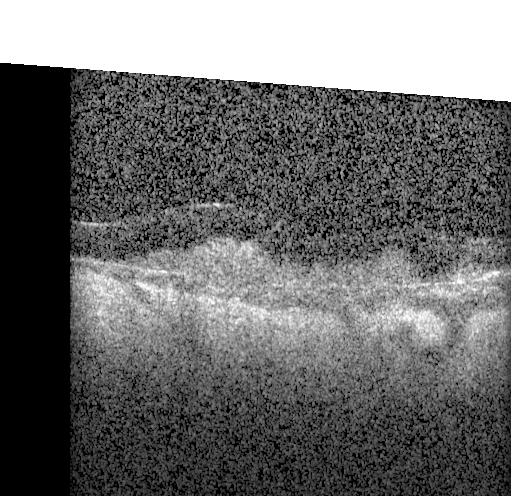 Acquired on a Heidelberg Spectralis. OCT line scan
Diagnosis: a choroidal neovascular membrane.